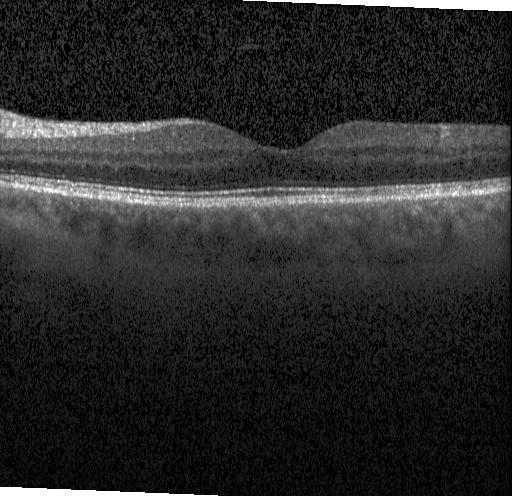
Heidelberg Spectralis OCT system · OCT line scan. No evidence of choroidal neovascularization, diabetic macular edema, or drusen.